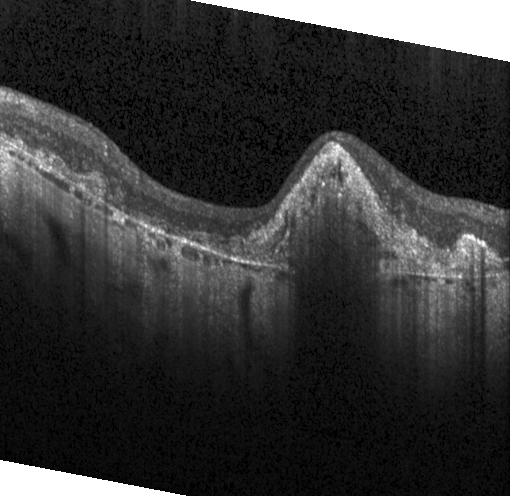 OCT finding: CNV.